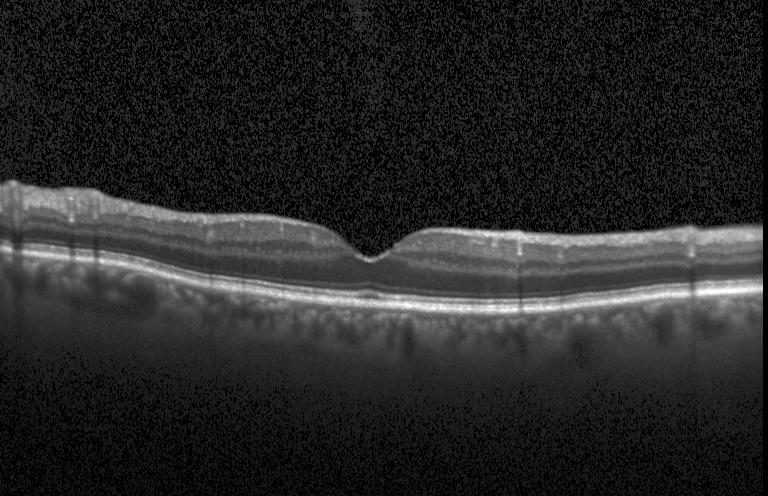
OCT B-scan, spectral-domain optical coherence tomography. Impression: neither choroidal neovascularization, diabetic macular edema, nor drusen.